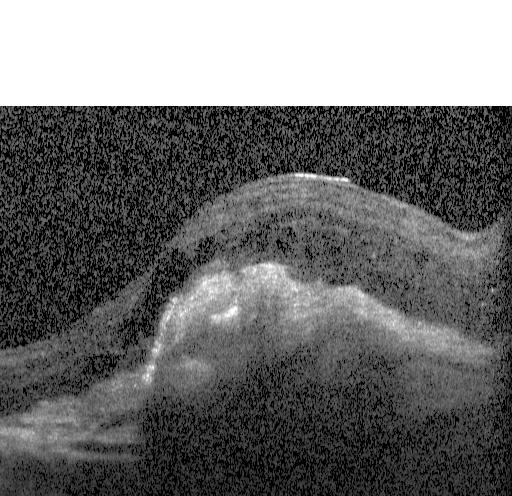 Spectral-domain OCT. Fovea-centered. Instrument: Heidelberg Spectralis. OCT line scan
The scan shows a choroidal neovascular membrane.